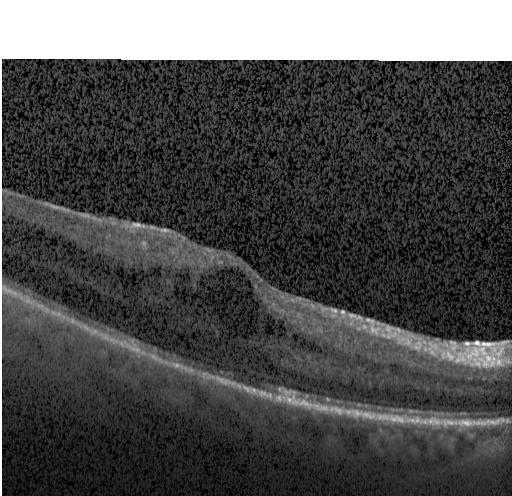 Optical coherence tomography B-scan; horizontal scan through the fovea. The scan shows DME.